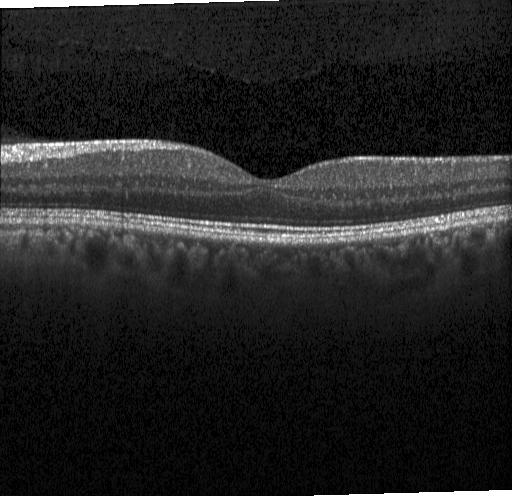

Spectral-domain optical coherence tomography; retinal OCT B-scan; macular scan; Heidelberg Spectralis
Macular OCT: no choroidal neovascularization, diabetic macular edema, or drusen.